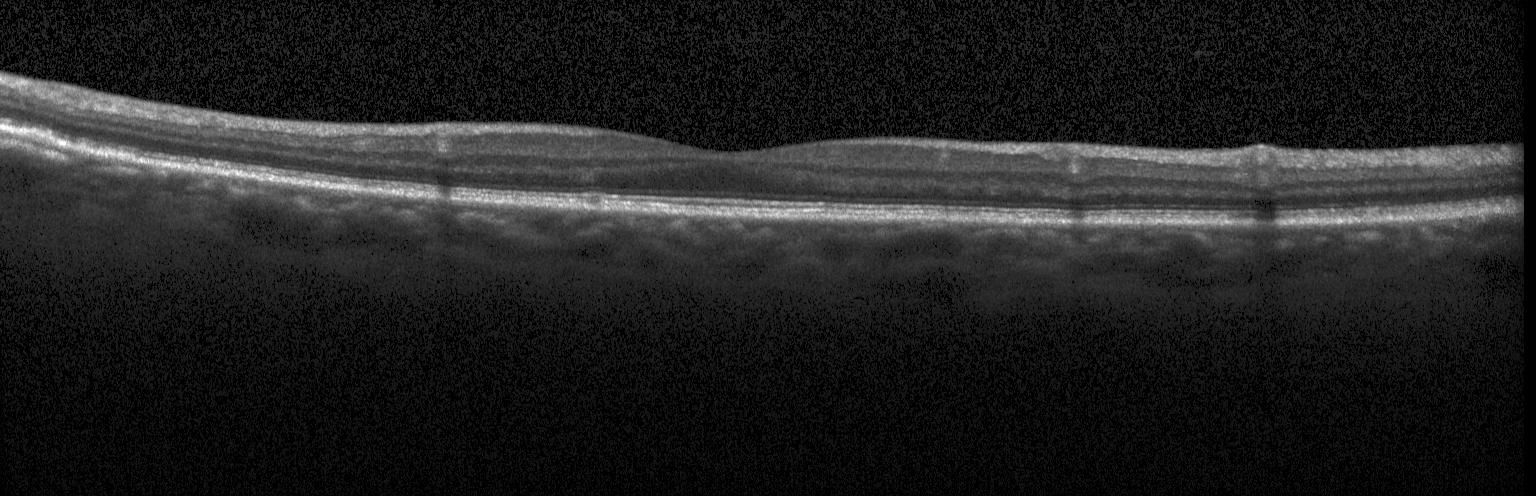
Optical coherence tomography scan · fovea-centered — No choroidal neovascularization, no diabetic macular edema, and no drusen.